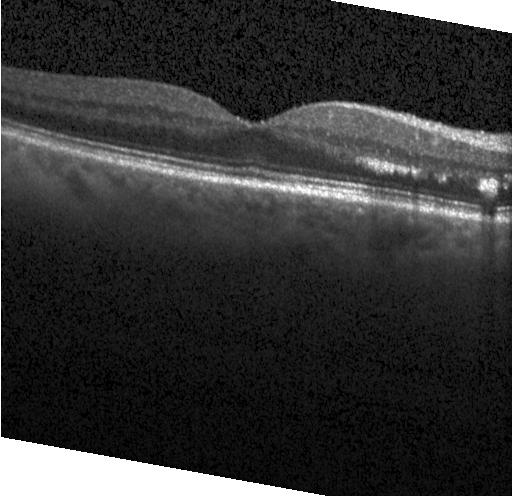 Spectral-domain OCT, fovea-centered, OCT line scan, Heidelberg Spectralis OCT system
Diagnosis: no choroidal neovascularization, diabetic macular edema, or drusen.